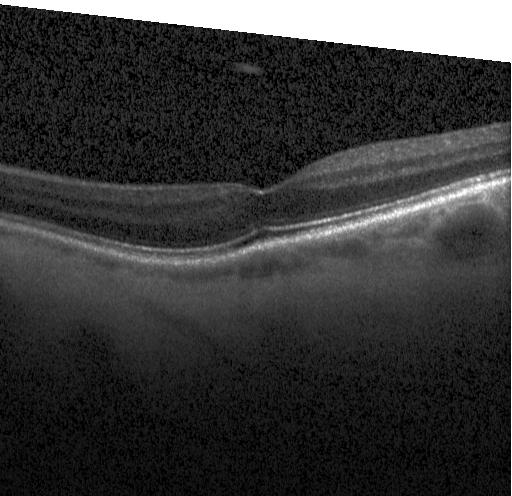

Retinal OCT cross-section showing no choroidal neovascularization, no diabetic macular edema, and no drusen.